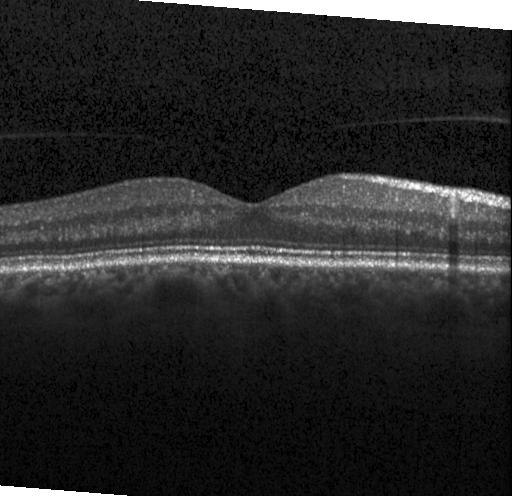 Horizontal scan through the fovea, retinal OCT B-scan, spectral-domain optical coherence tomography — Finding: no choroidal neovascularization, no diabetic macular edema, and no drusen.